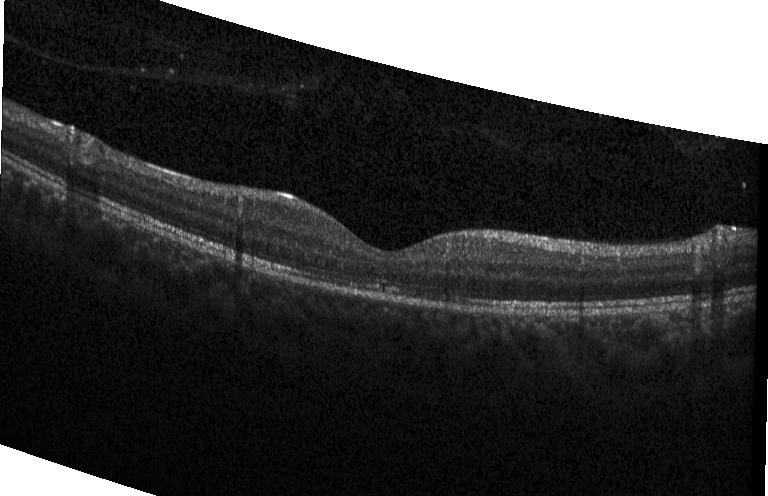 Retinal OCT cross-section, spectral-domain optical coherence tomography — Diagnosis: no evidence of choroidal neovascularization, diabetic macular edema, or drusen.